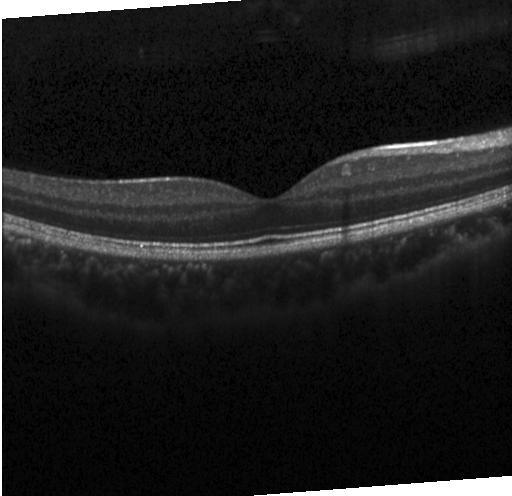
Acquired on a Heidelberg Spectralis, spectral-domain optical coherence tomography, OCT B-scan.
Assessment: no evidence of CNV, DME, or drusen.